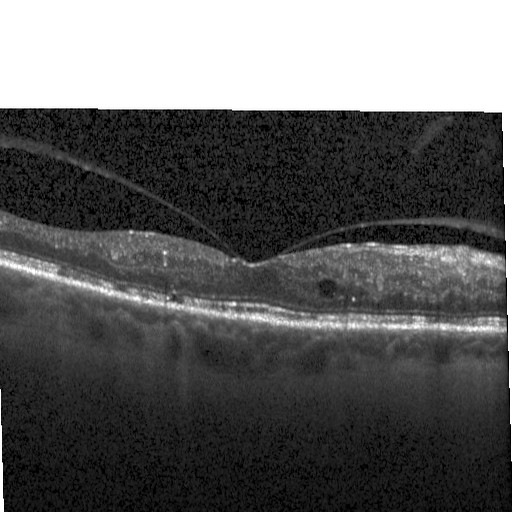
Instrument: Heidelberg Spectralis · fovea-centered · optical coherence tomography scan.
Dx: diabetic macular edema (DME).